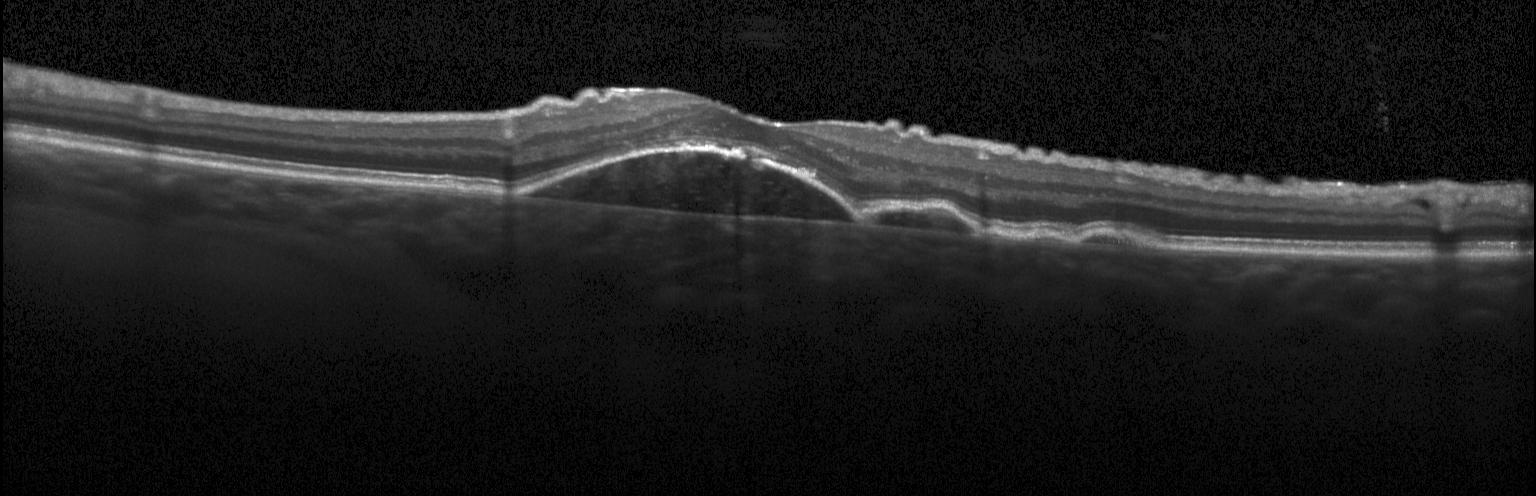

OCT line scan.
Impression: a choroidal neovascular membrane.